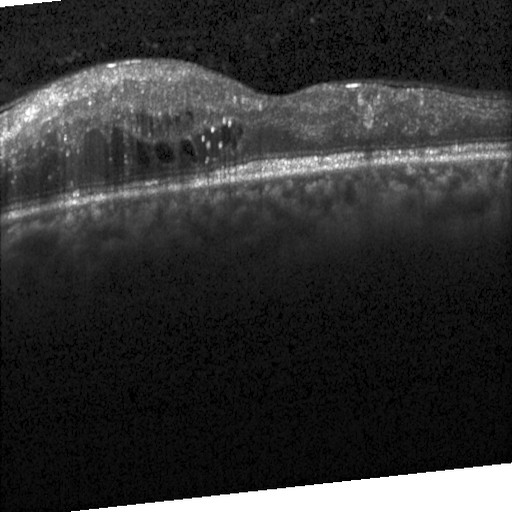

Diabetic macular edema (DME).